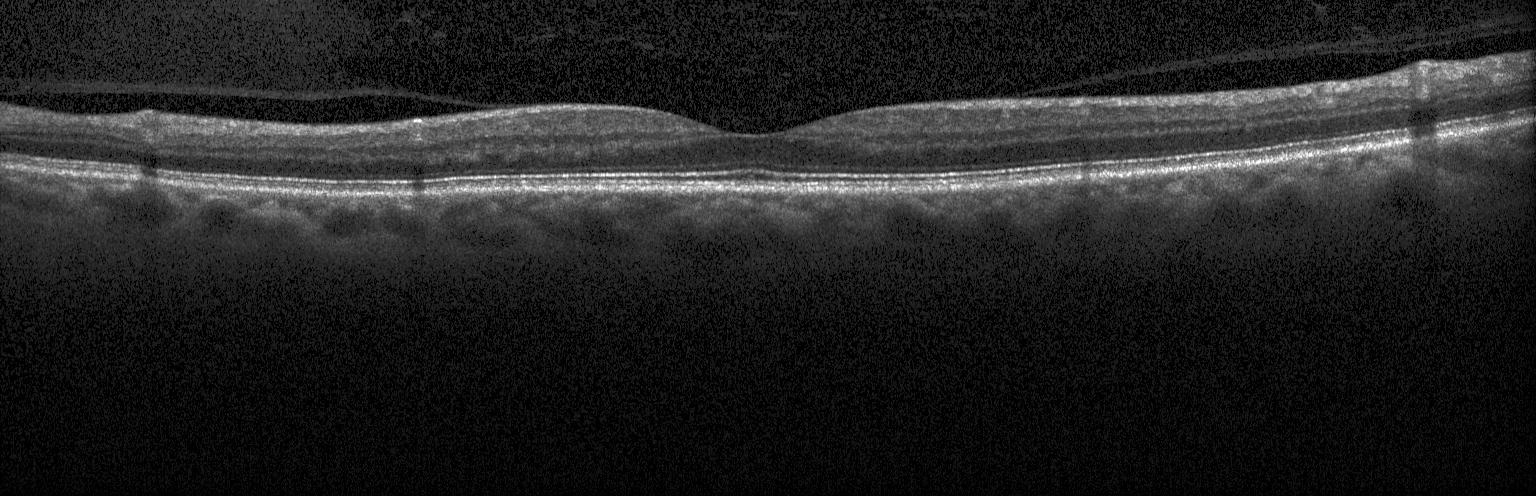

Heidelberg Spectralis · retinal OCT B-scan · macular scan
The scan shows no choroidal neovascularization, diabetic macular edema, or drusen.